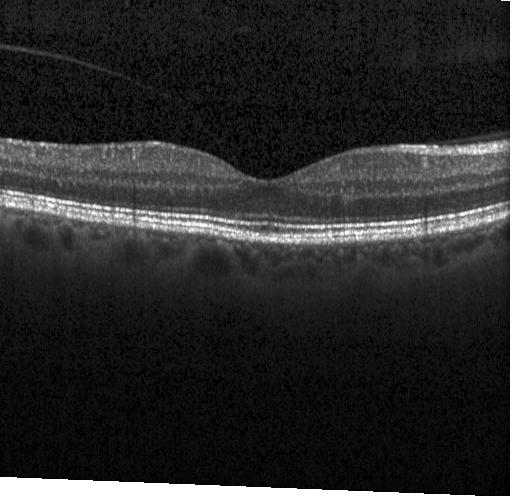

Macular OCT demonstrating neither CNV, DME, nor drusen.